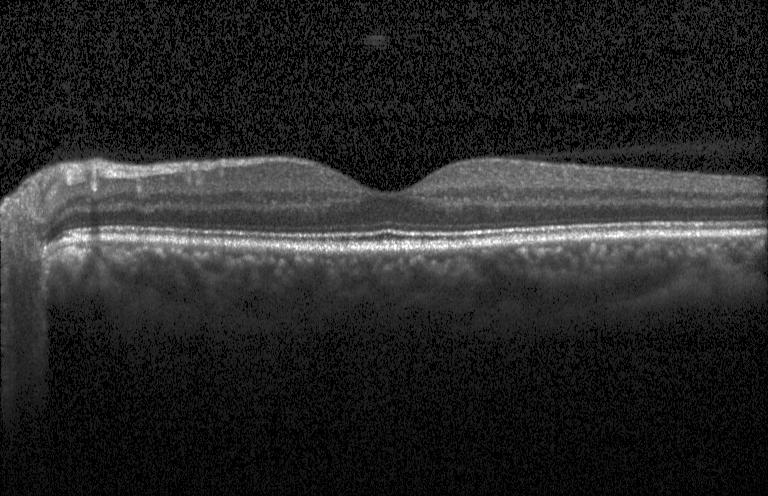
No choroidal neovascularization, no diabetic macular edema, and no drusen.